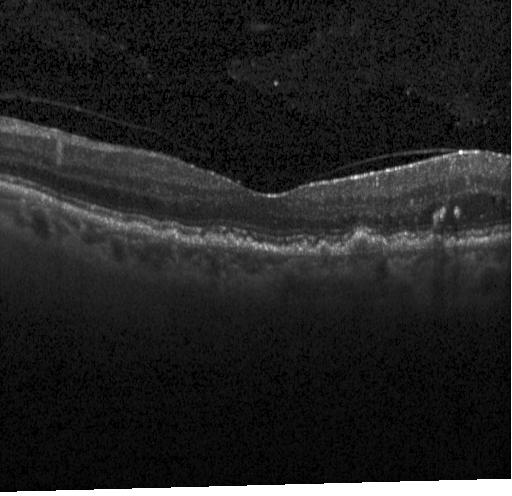 Spectral-domain OCT, instrument: Heidelberg Spectralis, retinal OCT B-scan
Assessment: CNV.